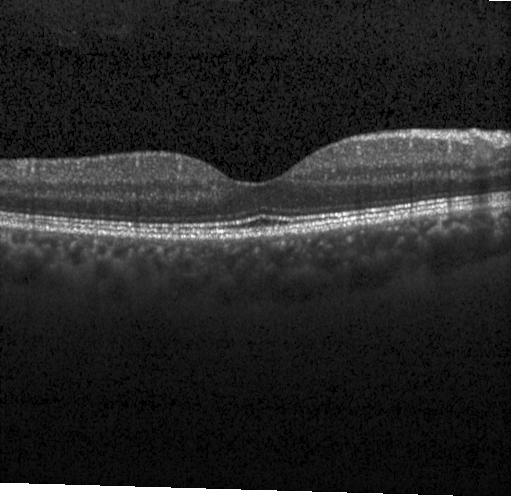
Finding: no evidence of CNV, DME, or drusen.